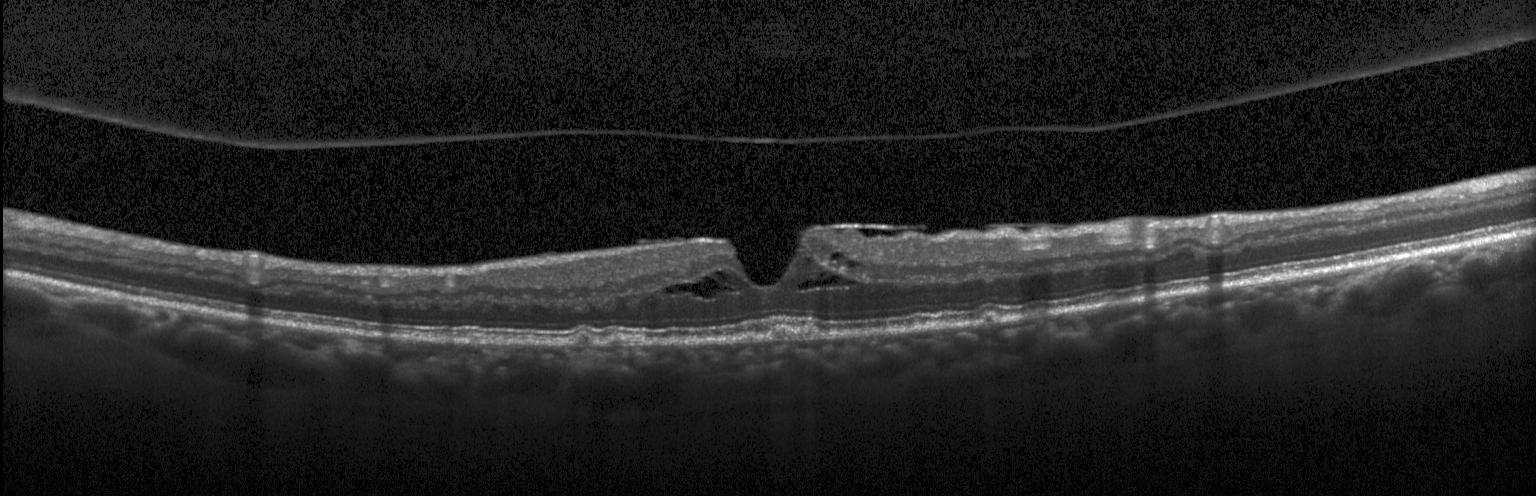 Dx: multiple drusen.